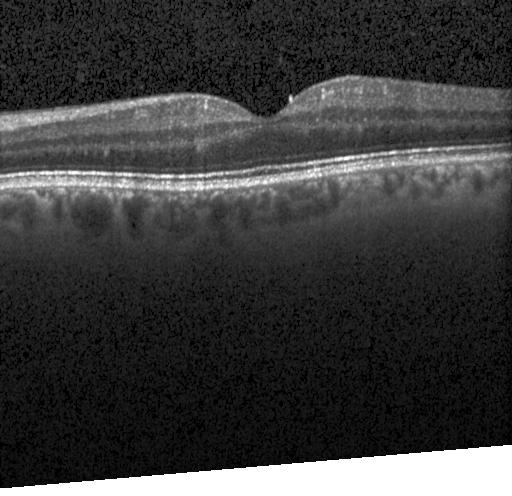
Fovea-centered; acquired on a Heidelberg Spectralis; optical coherence tomography scan. Finding: no CNV, no DME, and no drusen.